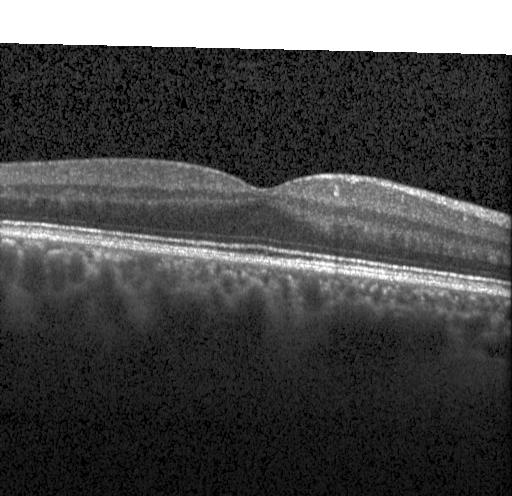

Macular OCT: no evidence of CNV, DME, or drusen.